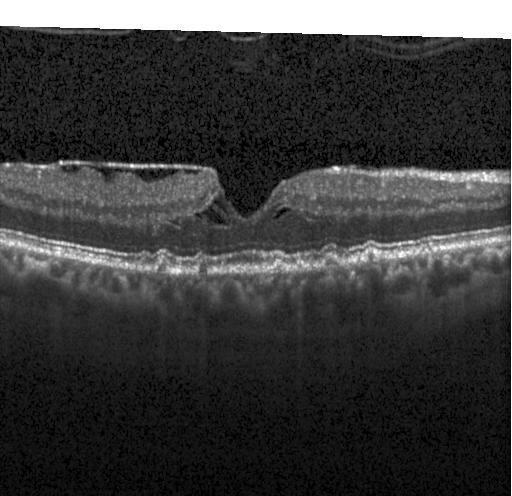

Macular OCT: drusen.